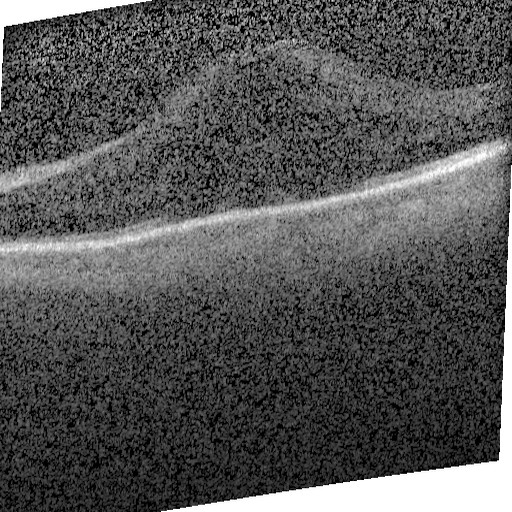
OCT scan showing diabetic macular edema.